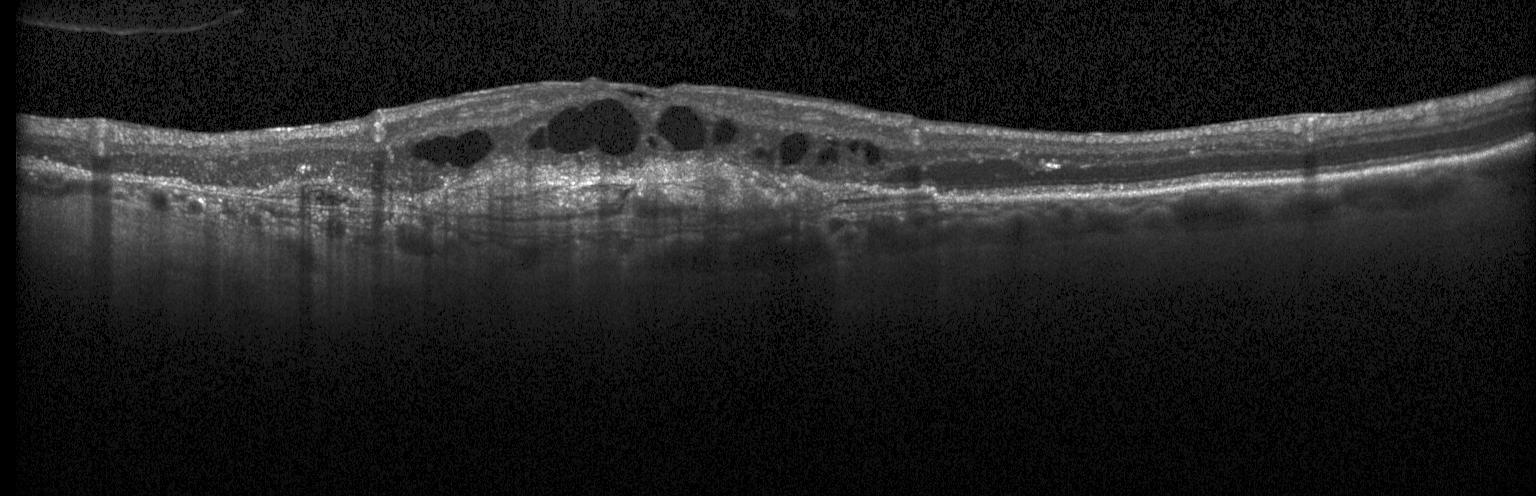

OCT line scan. OCT finding: choroidal neovascularization (CNV).